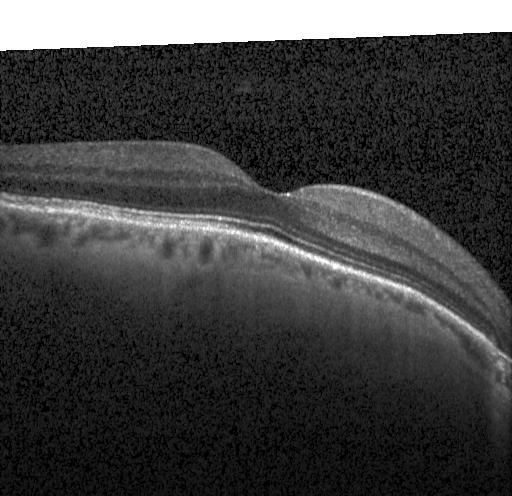

Retinal OCT cross-section showing no choroidal neovascularization, no diabetic macular edema, and no drusen.